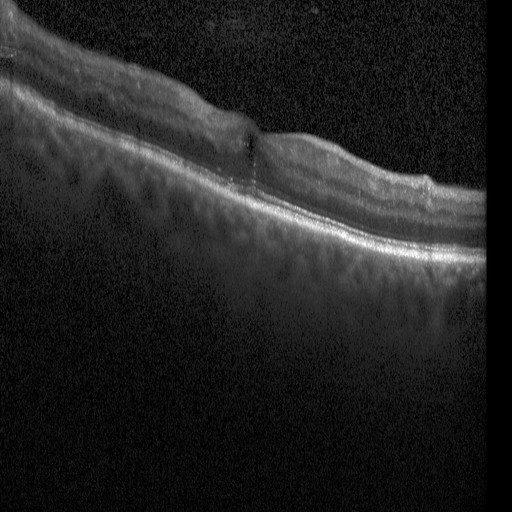

OCT scan showing diabetic macular edema (DME).